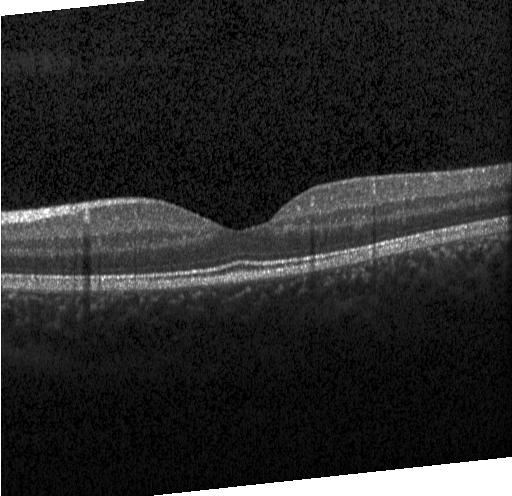
Retinal OCT cross-section.
The scan shows no choroidal neovascularization, no diabetic macular edema, and no drusen.